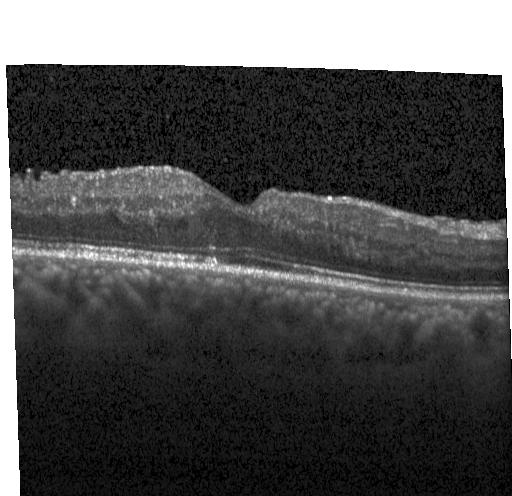
Fovea-centered; SD-OCT; retinal OCT B-scan; Heidelberg Spectralis. This B-scan demonstrates diabetic macular edema.